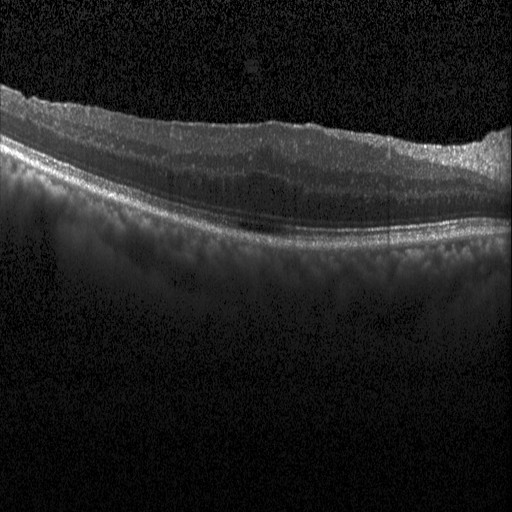

Spectral-domain OCT · retinal OCT B-scan.
The scan shows diabetic macular edema.